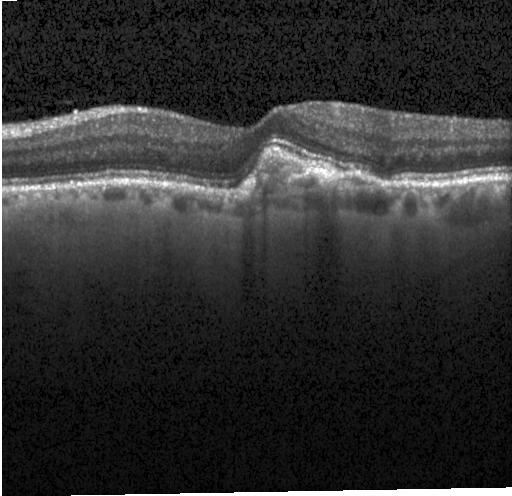
Assessment: a choroidal neovascular membrane.